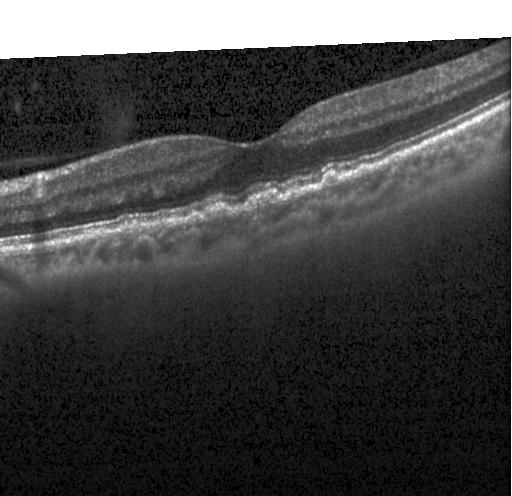

OCT line scan. OCT finding: sub-RPE drusenoid deposits.